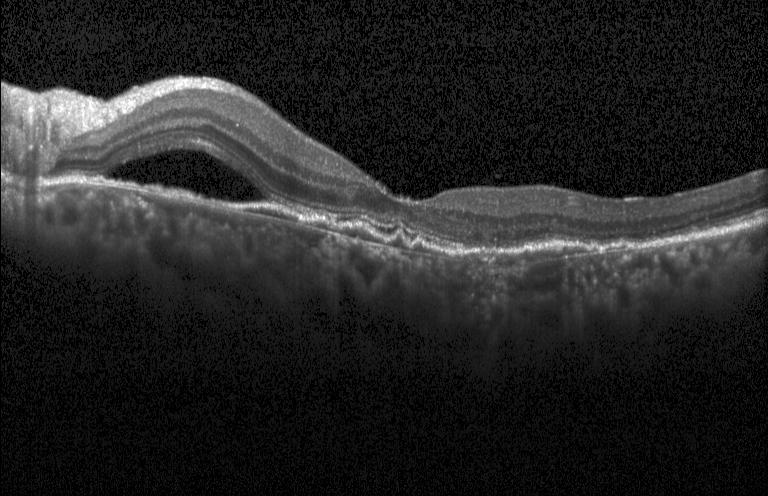 Macular OCT: a choroidal neovascular membrane.